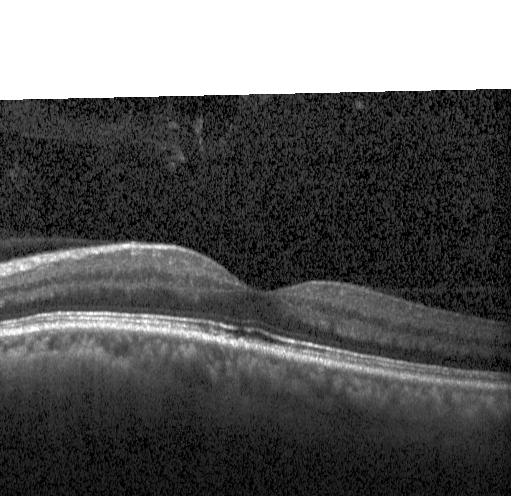
Fovea-centered; optical coherence tomography B-scan.
The scan shows no evidence of CNV, DME, or drusen.